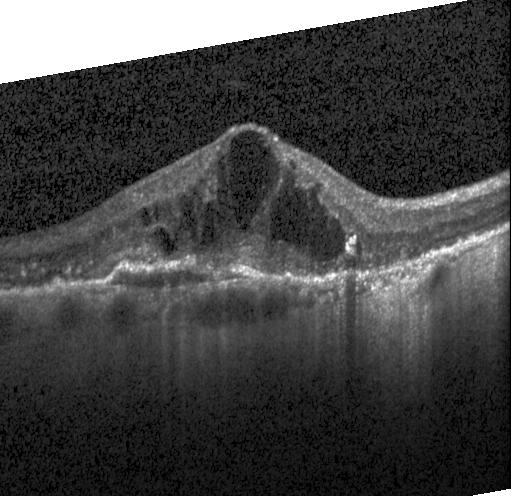 Diagnosis: choroidal neovascularization (CNV).